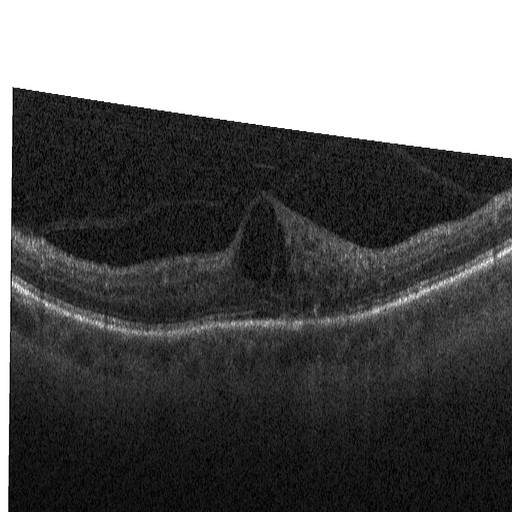
Dx: diabetic macular edema.